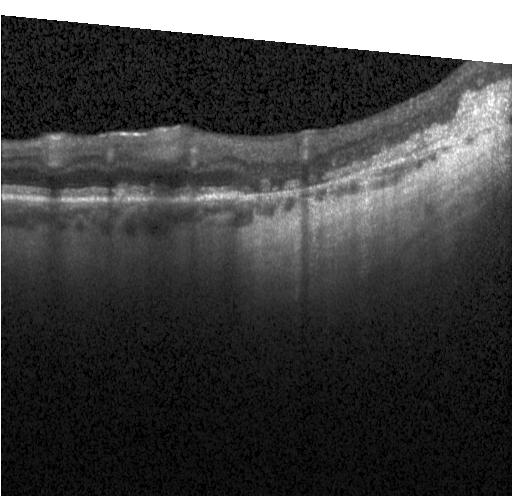

Macular OCT: a choroidal neovascular membrane.